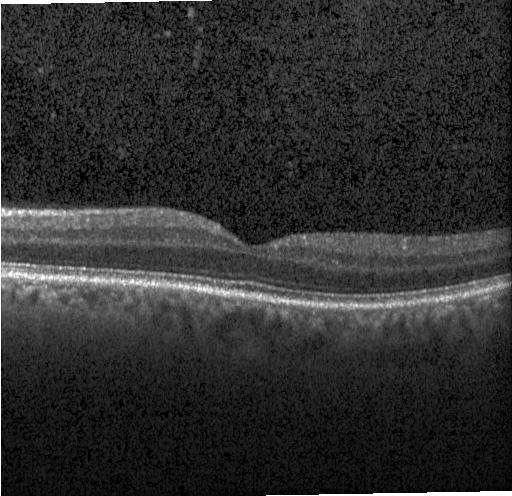 Spectral-domain optical coherence tomography, OCT B-scan, macular scan, Heidelberg Spectralis
OCT finding: no evidence of CNV, DME, or drusen.